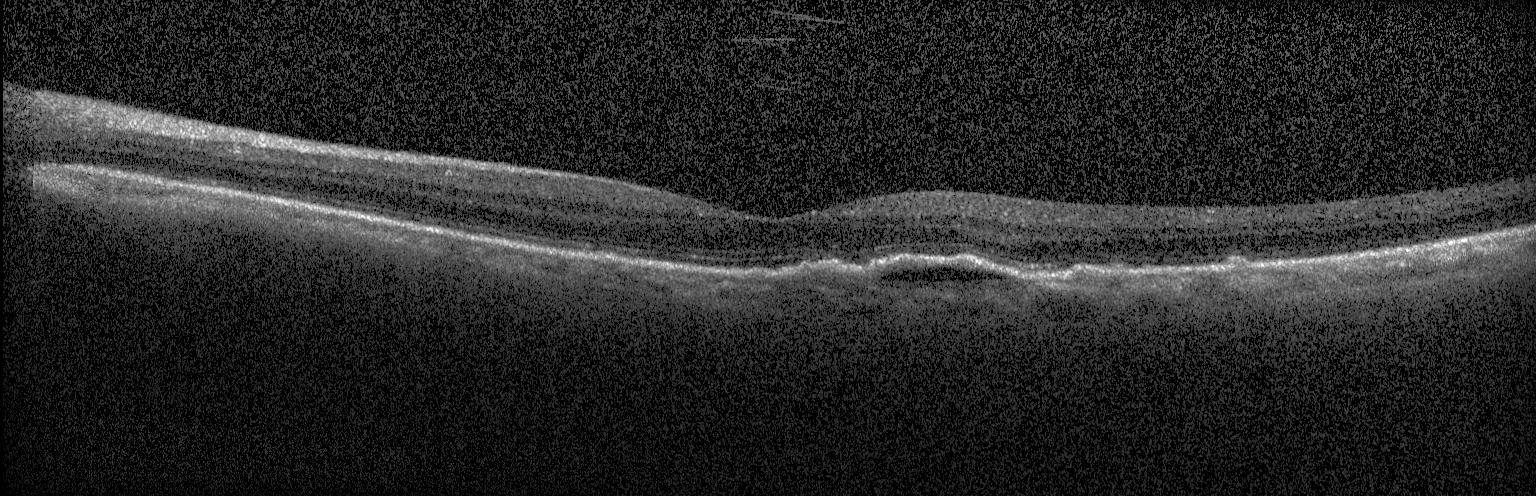

Retinal OCT cross-section — Macular OCT: a choroidal neovascular membrane.